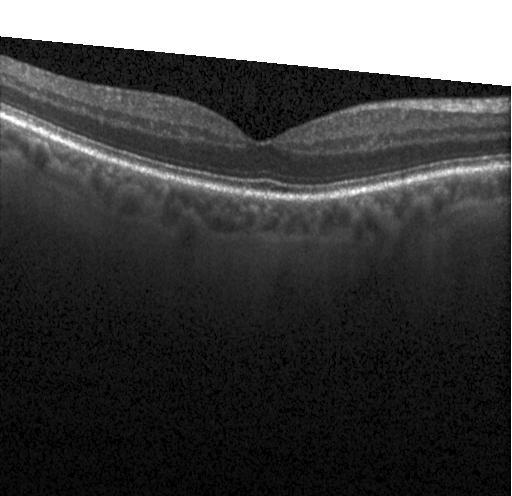

Spectral-domain OCT. Centered on the fovea. OCT B-scan.
The scan shows no CNV, DME, or drusen.